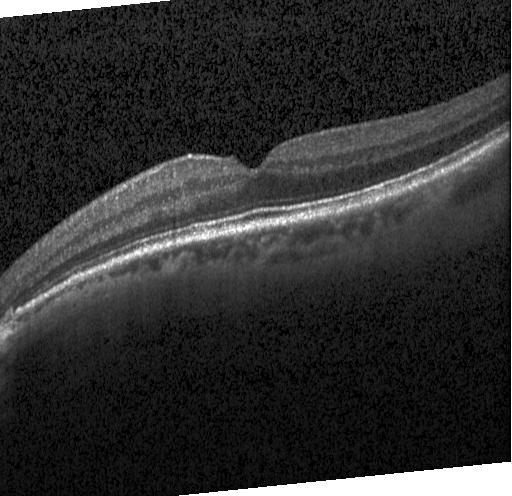
Heidelberg Spectralis. Spectral-domain OCT. OCT line scan
Impression: no choroidal neovascularization, diabetic macular edema, or drusen.